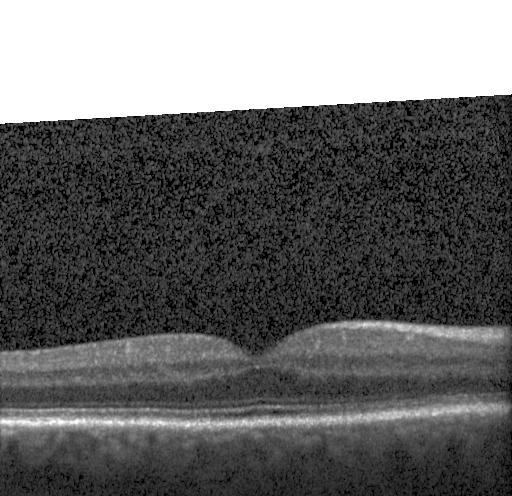

Spectral-domain optical coherence tomography, centered on the fovea, instrument: Heidelberg Spectralis, optical coherence tomography scan — Macular OCT: no choroidal neovascularization, no diabetic macular edema, and no drusen.